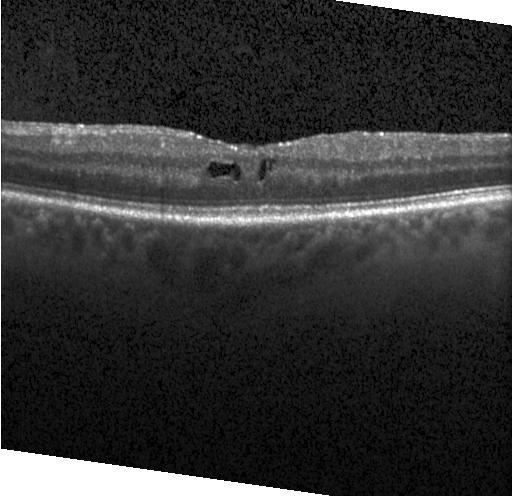
This B-scan demonstrates diabetic macular edema.